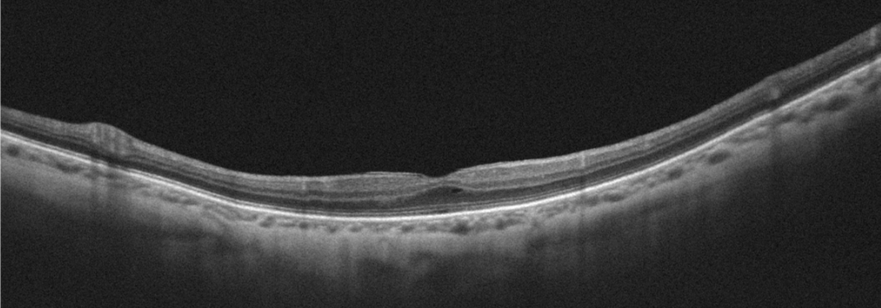 This B-scan demonstrates VID.